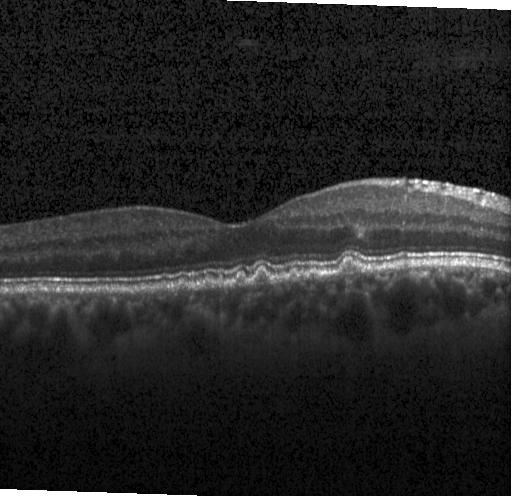
Macular OCT: sub-RPE drusenoid deposits.